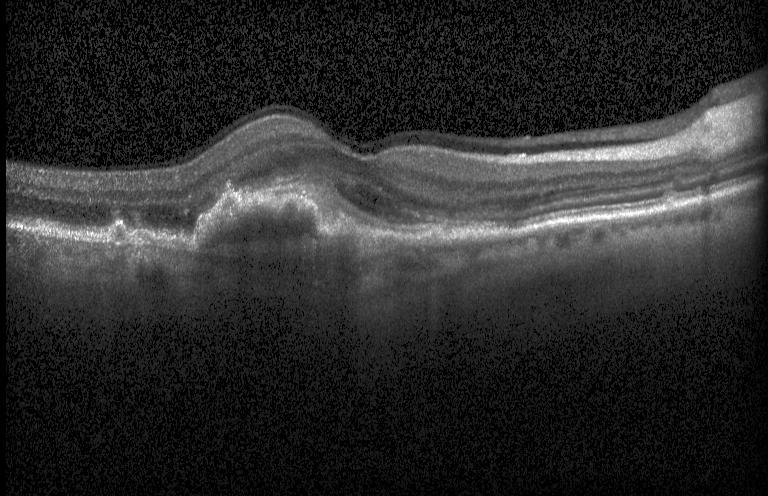 Spectral-domain optical coherence tomography, retinal OCT B-scan, horizontal scan through the fovea
This B-scan demonstrates a choroidal neovascular membrane.